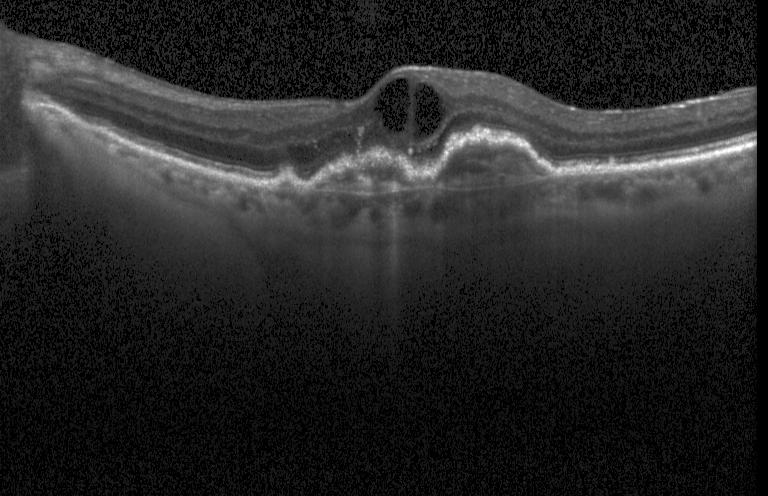
Spectral-domain optical coherence tomography, OCT B-scan, Heidelberg Spectralis, macular scan
Diagnosis: CNV.